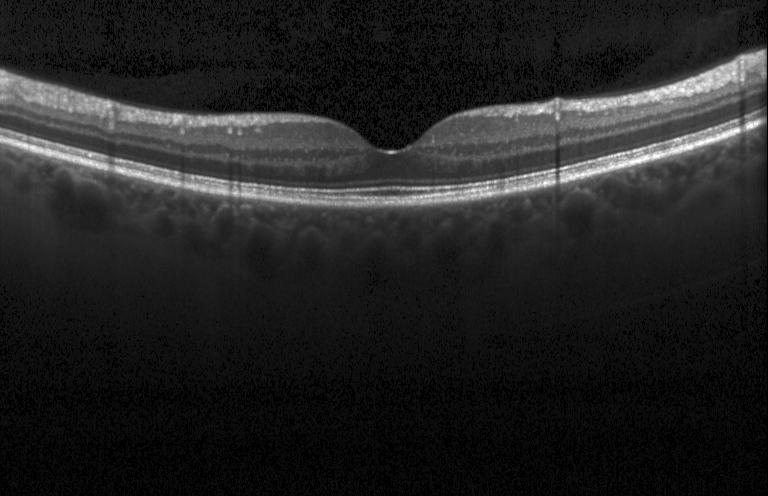
The scan shows no choroidal neovascularization, no diabetic macular edema, and no drusen.